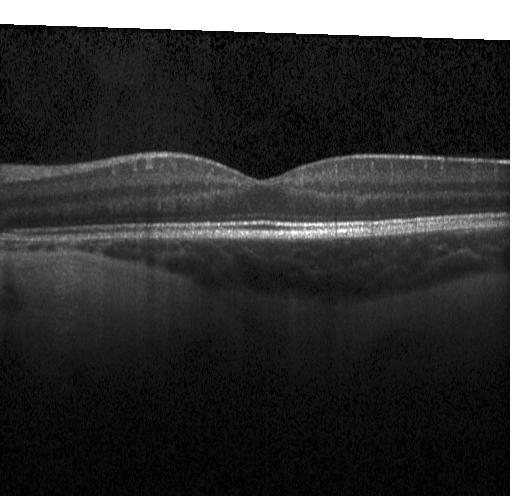

Optical coherence tomography scan — Diagnosis: neither CNV, DME, nor drusen.